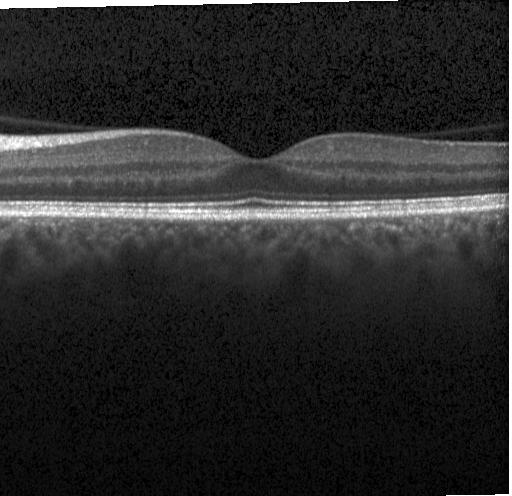

Spectral-domain OCT · retinal OCT B-scan. Impression: no CNV, no DME, and no drusen.